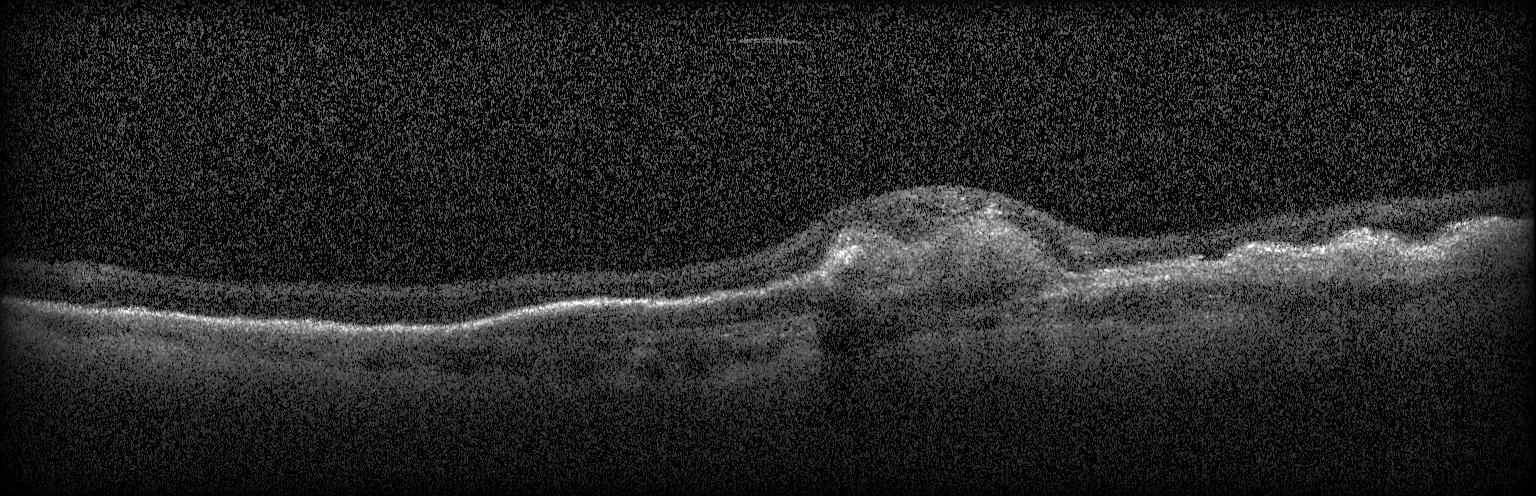
Acquired on a Heidelberg Spectralis, OCT B-scan, SD-OCT.
CNV.